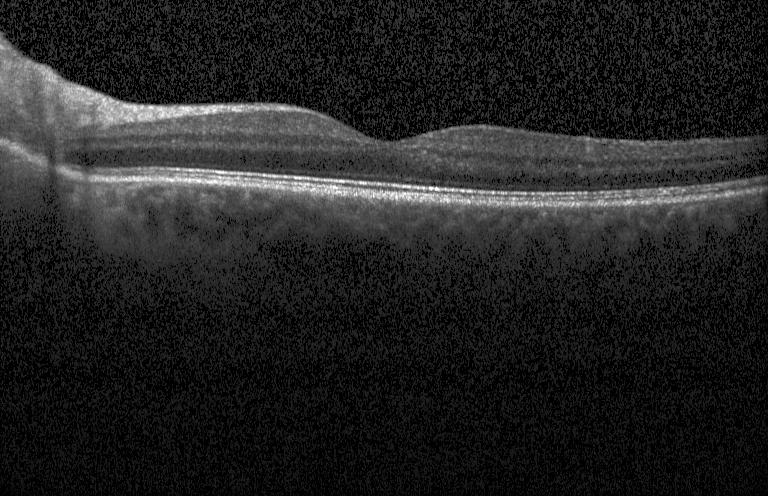
This B-scan demonstrates no evidence of choroidal neovascularization, diabetic macular edema, or drusen.